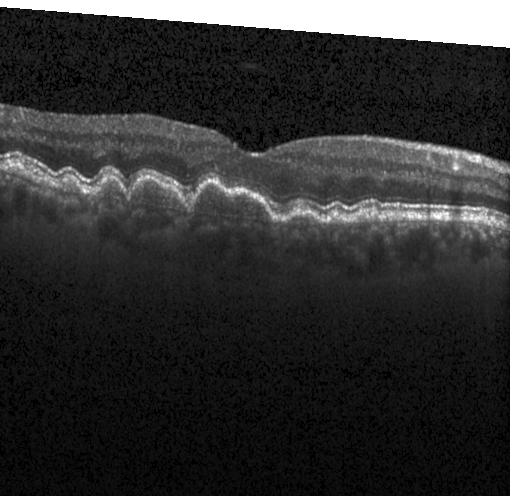 Fovea-centered. Spectral-domain OCT. Instrument: Heidelberg Spectralis. Optical coherence tomography B-scan — Diagnosis: drusen.